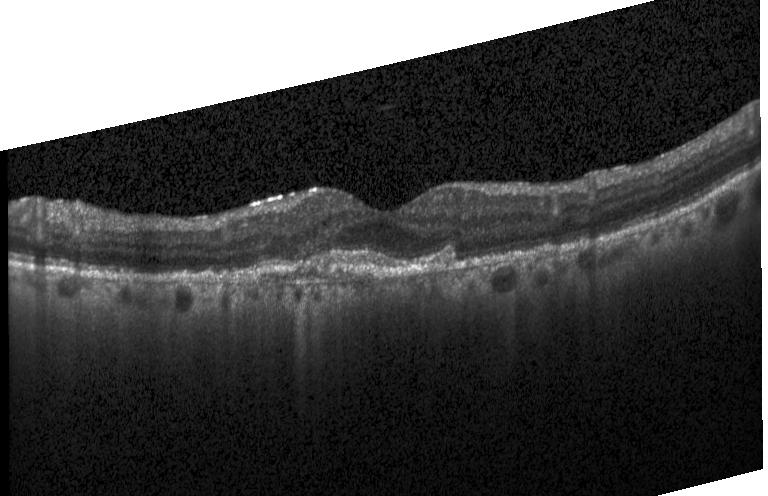 Fovea-centered · Heidelberg Spectralis OCT system · OCT B-scan
Finding: a choroidal neovascular membrane.